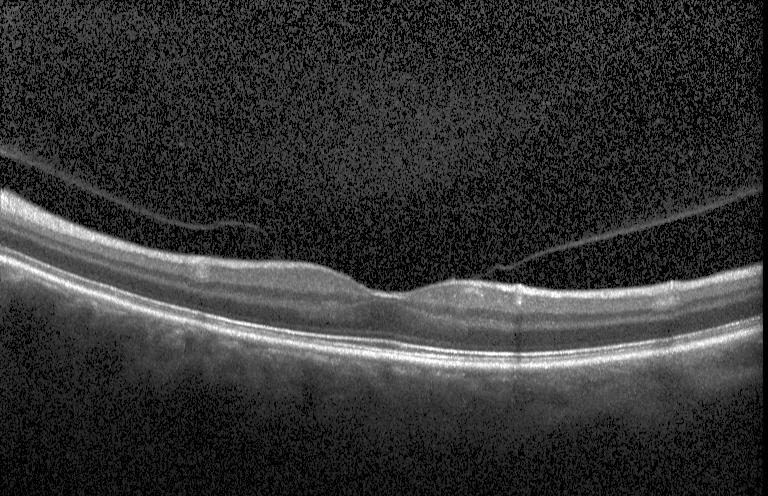 Heidelberg Spectralis OCT system · spectral-domain OCT · optical coherence tomography B-scan.
Finding: neither CNV, DME, nor drusen.